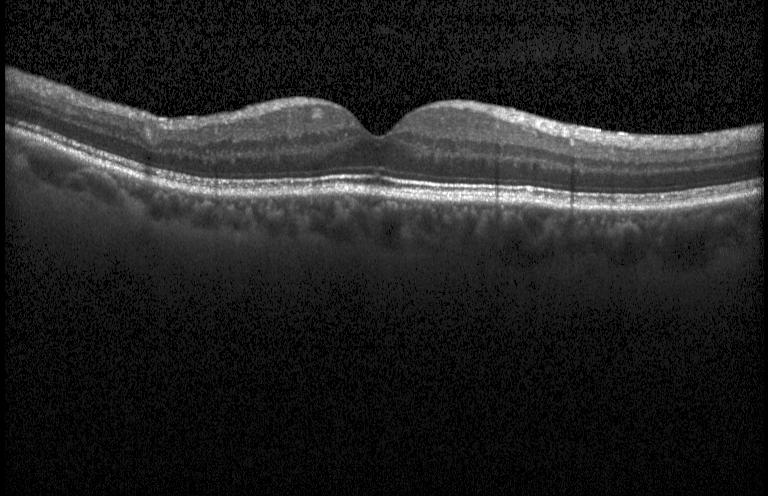 Impression: no choroidal neovascularization, no diabetic macular edema, and no drusen.